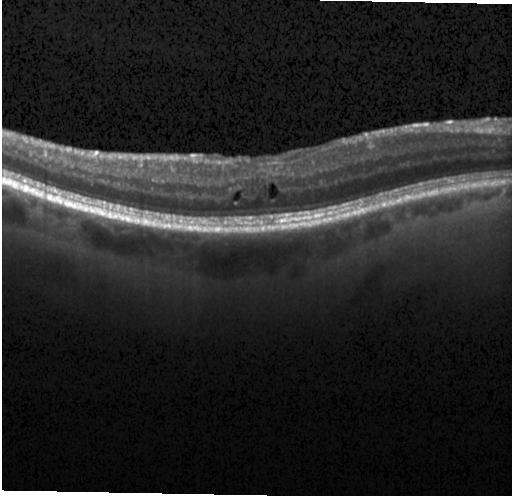

Instrument: Heidelberg Spectralis · OCT B-scan · macular scan · spectral-domain OCT. Diagnosis: DME.